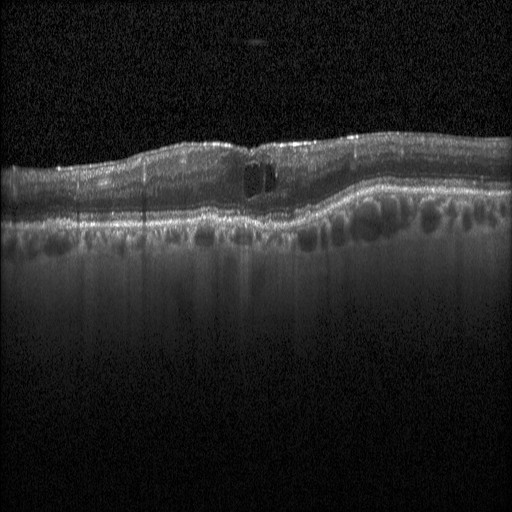
Dx: diabetic macular edema.